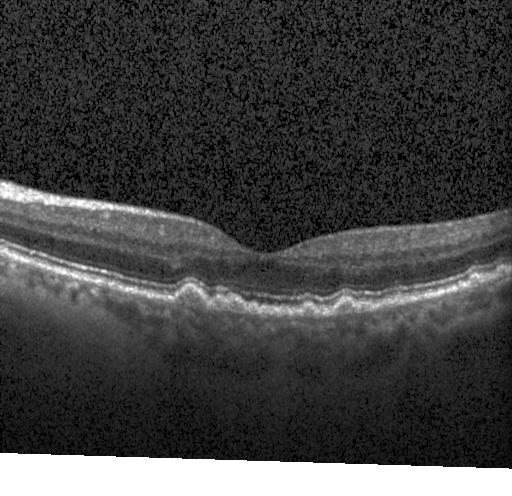

Through the macula; OCT B-scan; acquired on a Heidelberg Spectralis
Finding: drusen.